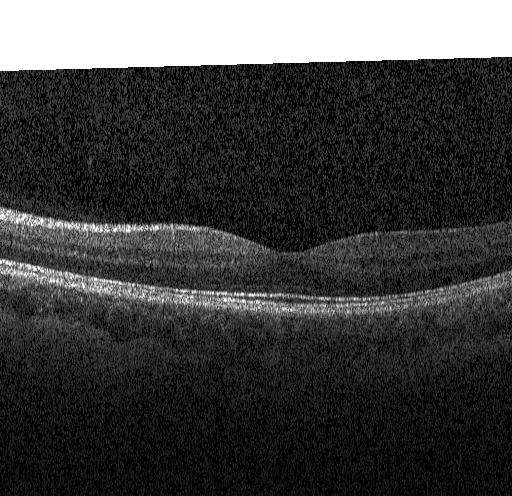

Macular scan · OCT B-scan · spectral-domain OCT — This B-scan demonstrates no evidence of choroidal neovascularization, diabetic macular edema, or drusen.